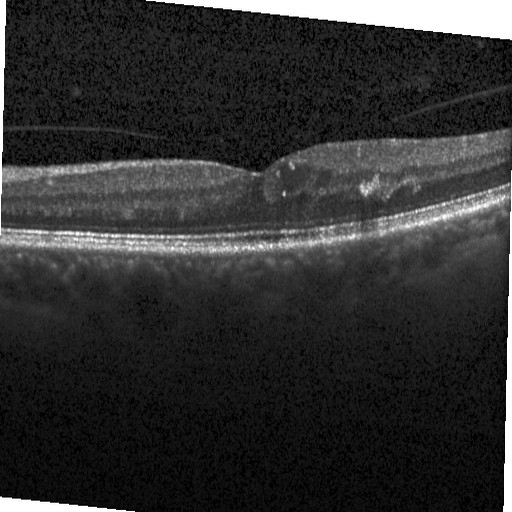
Spectral-domain OCT. OCT B-scan. Acquired on a Heidelberg Spectralis.
This B-scan demonstrates DME.